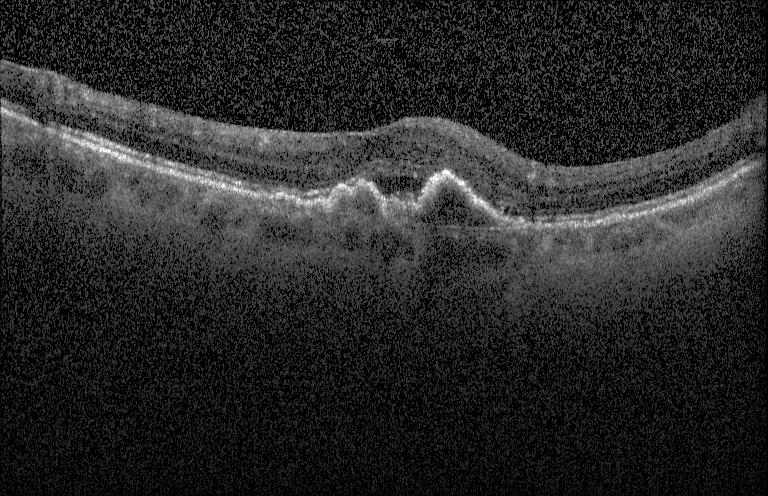

Fovea-centered; OCT line scan; spectral-domain OCT; Heidelberg Spectralis
A choroidal neovascular membrane.